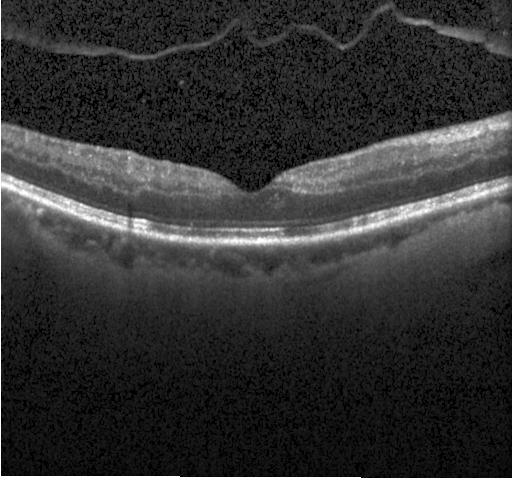 Instrument: Heidelberg Spectralis. Spectral-domain optical coherence tomography. Retinal OCT cross-section.
Macular OCT: neither choroidal neovascularization, diabetic macular edema, nor drusen.